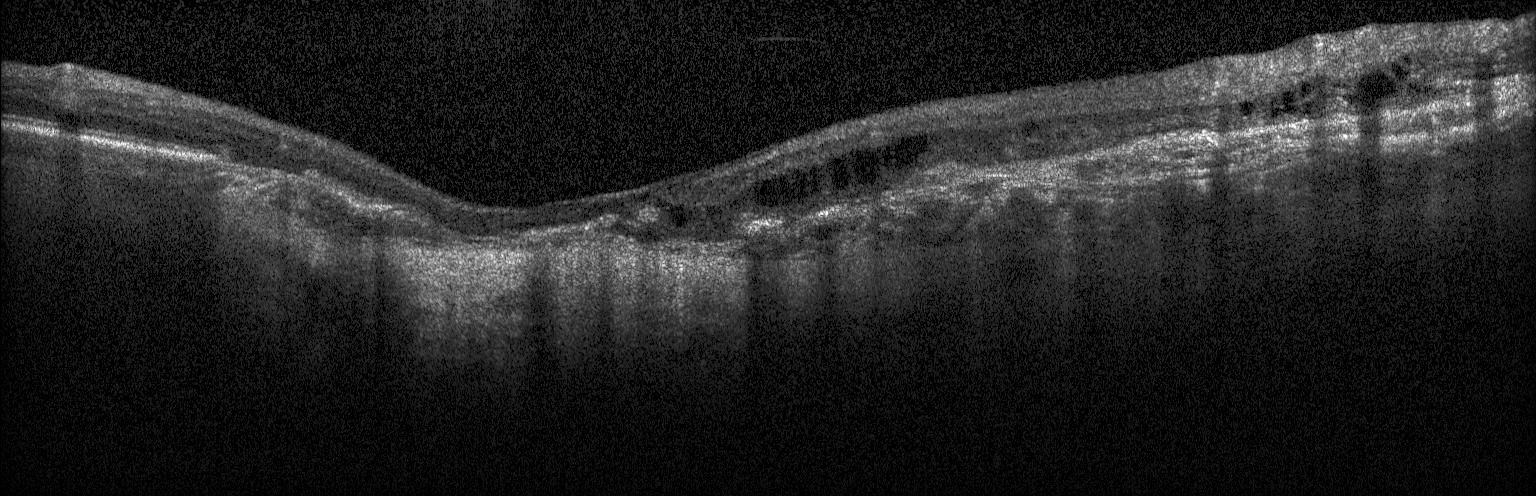
Macular OCT: a choroidal neovascular membrane.